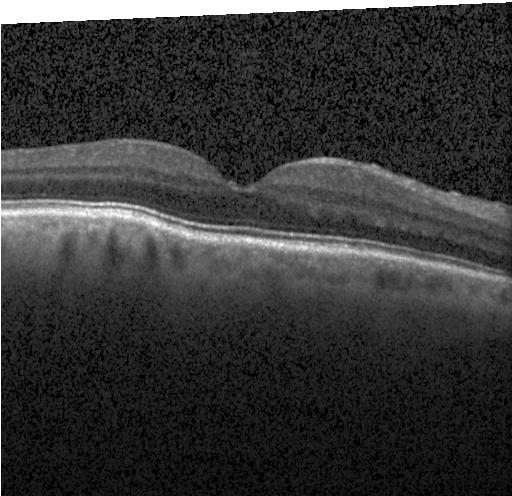

Through the macula · optical coherence tomography B-scan · spectral-domain OCT · acquired on a Heidelberg Spectralis — Dx: no evidence of choroidal neovascularization, diabetic macular edema, or drusen.